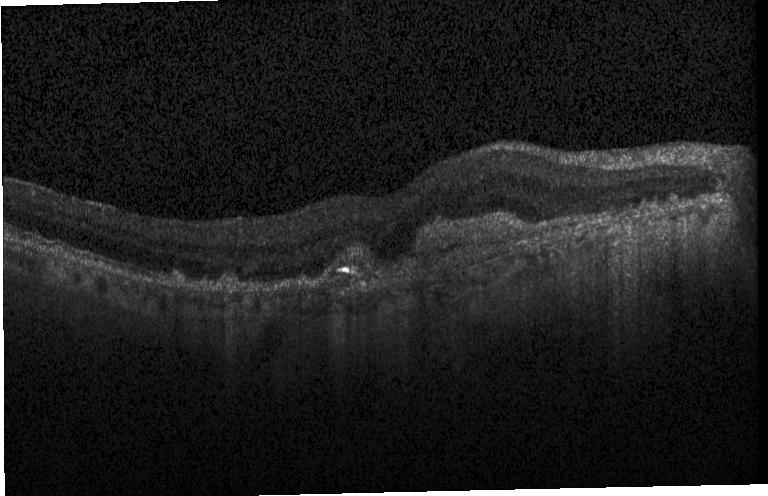

Retinal OCT cross-section. Heidelberg Spectralis OCT system
Finding: choroidal neovascularization (CNV).